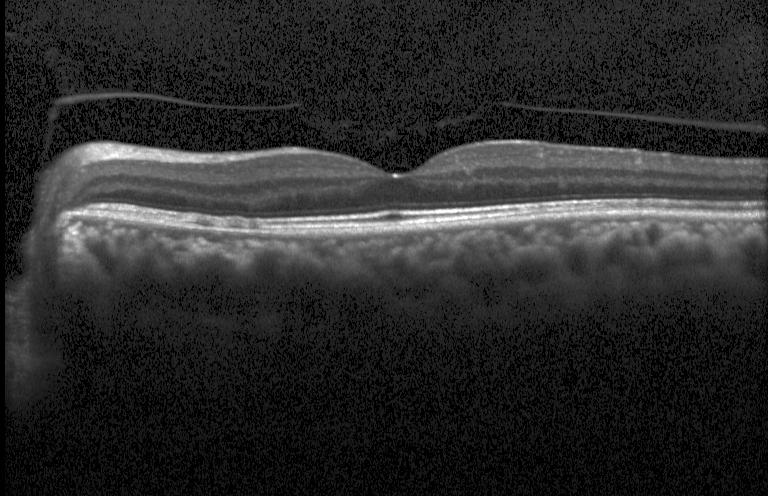
Dx: no choroidal neovascularization, no diabetic macular edema, and no drusen.